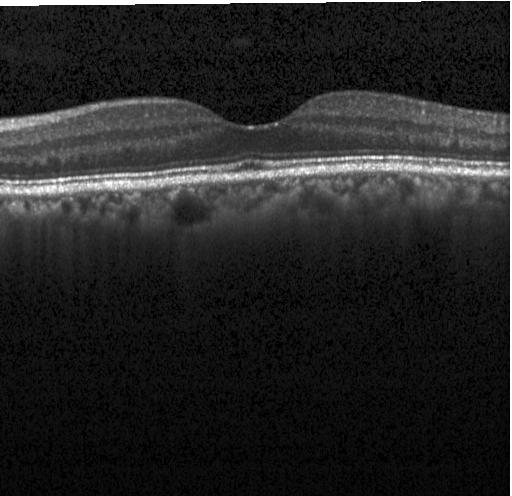
Diagnosis: no choroidal neovascularization, diabetic macular edema, or drusen.